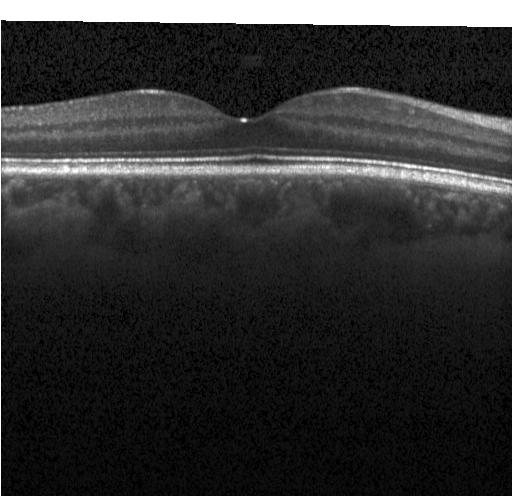 Retinal OCT B-scan; through the macula — This B-scan demonstrates no CNV, DME, or drusen.